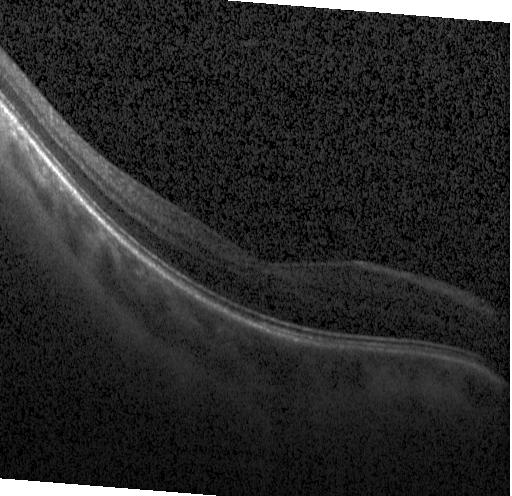
Heidelberg Spectralis, optical coherence tomography B-scan — Finding: neither choroidal neovascularization, diabetic macular edema, nor drusen.